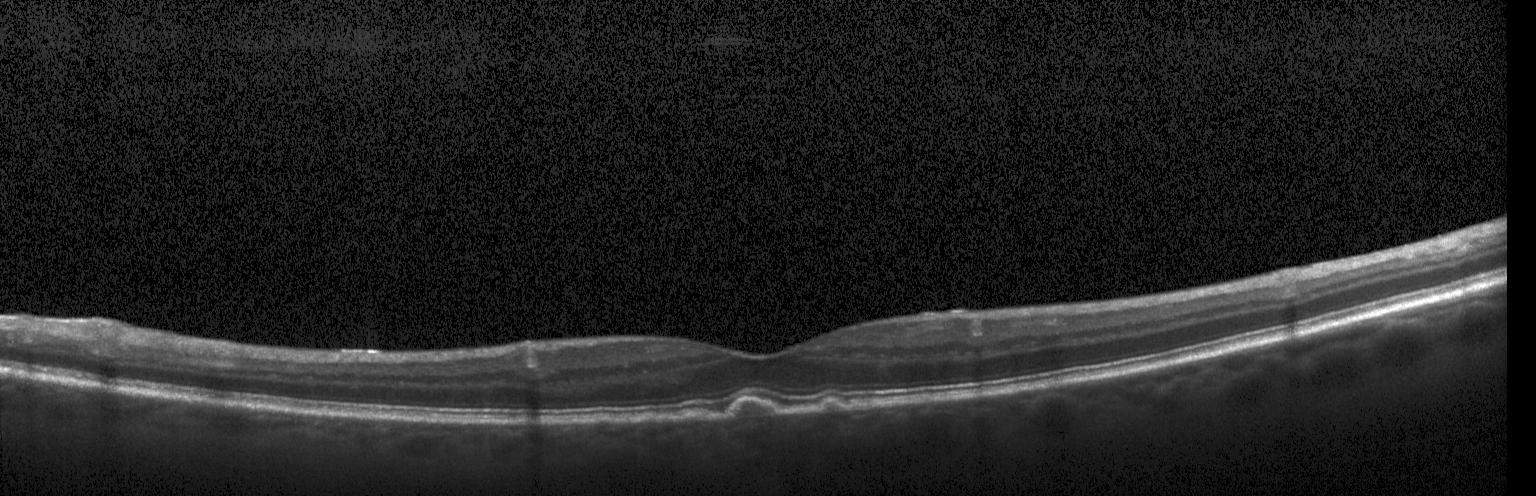 Through the macula; optical coherence tomography scan — Diagnosis: sub-RPE drusenoid deposits.